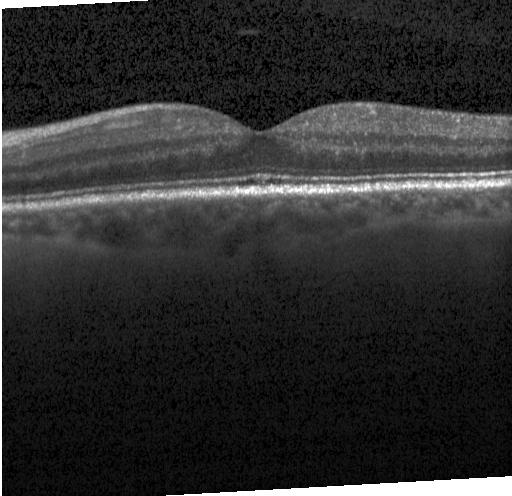
Retinal OCT B-scan; instrument: Heidelberg Spectralis.
Diagnosis: no choroidal neovascularization, no diabetic macular edema, and no drusen.